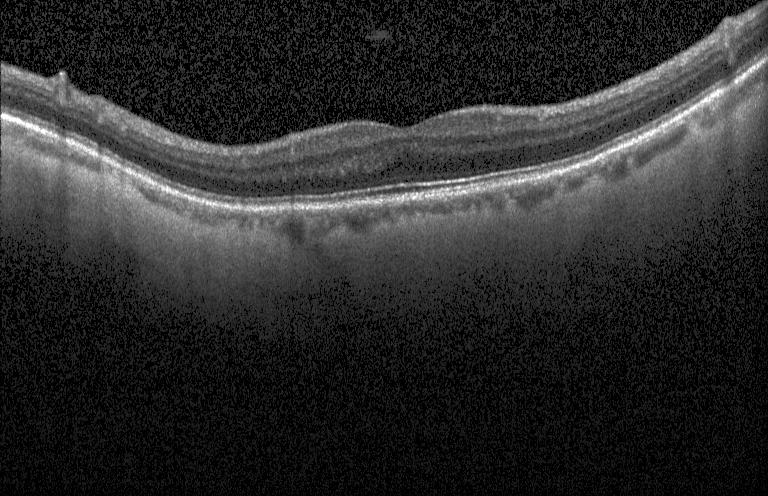 Impression: no choroidal neovascularization, no diabetic macular edema, and no drusen.